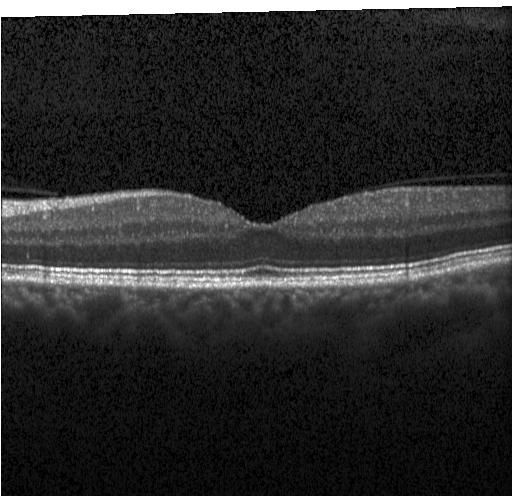 This B-scan demonstrates neither choroidal neovascularization, diabetic macular edema, nor drusen.